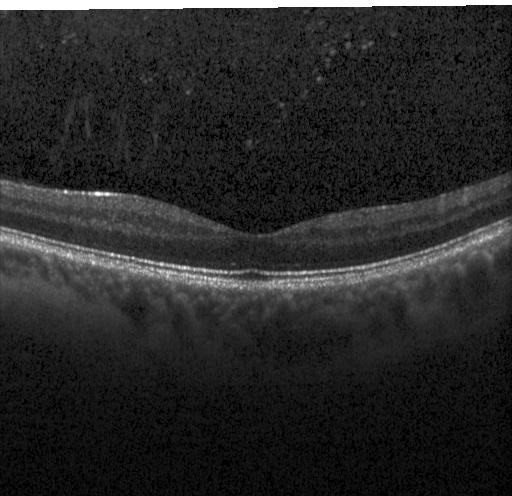
Dx: neither choroidal neovascularization, diabetic macular edema, nor drusen.